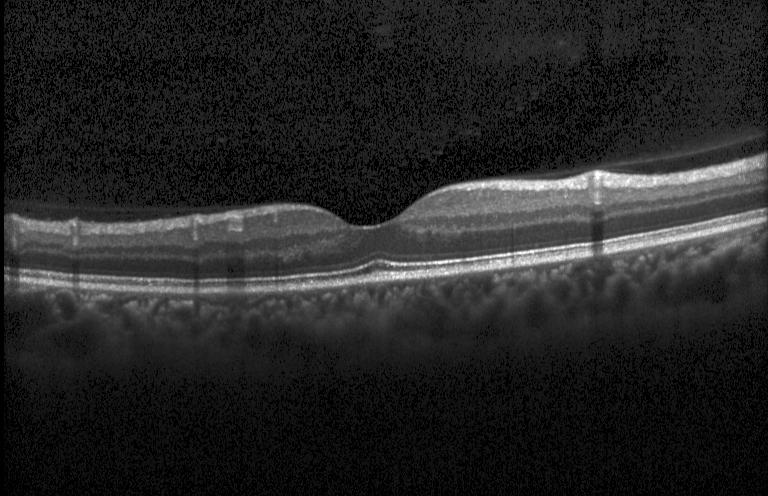

Centered on the fovea, OCT line scan. This B-scan demonstrates no choroidal neovascularization, diabetic macular edema, or drusen.